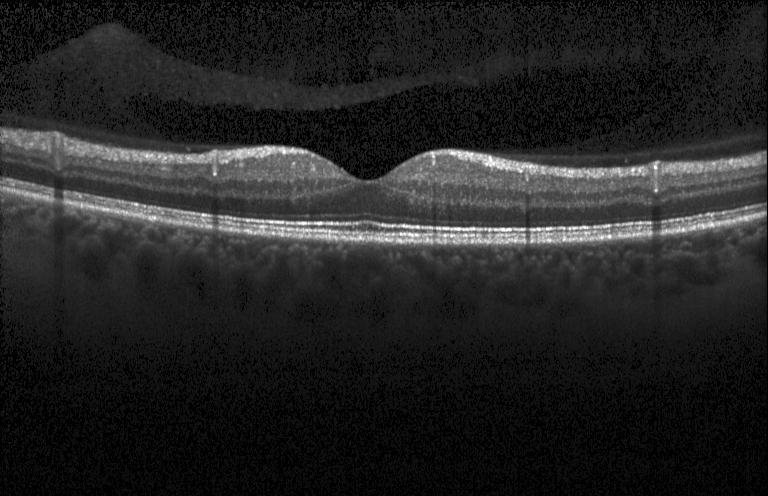
Diagnosis: no evidence of choroidal neovascularization, diabetic macular edema, or drusen.